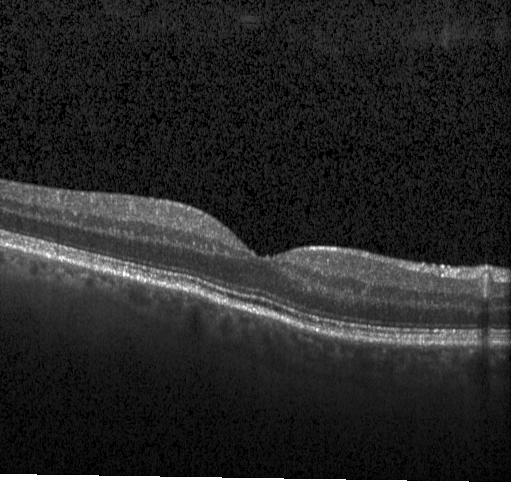

OCT scan showing no choroidal neovascularization, no diabetic macular edema, and no drusen.